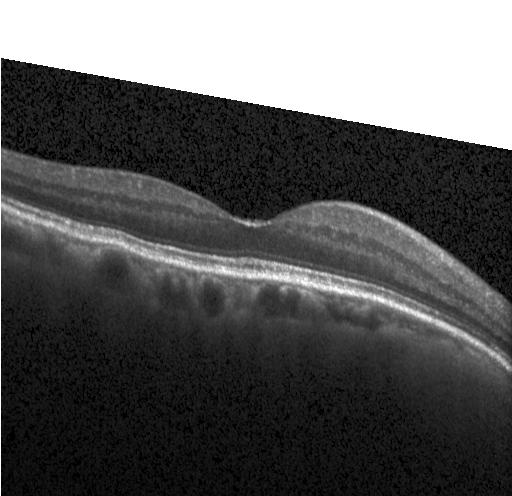
Finding: no evidence of choroidal neovascularization, diabetic macular edema, or drusen.